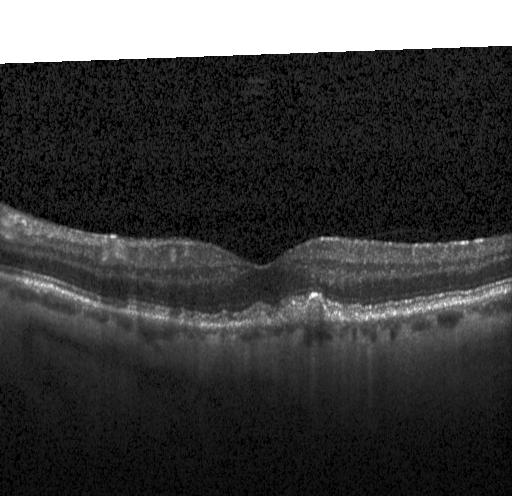

OCT finding: drusen.